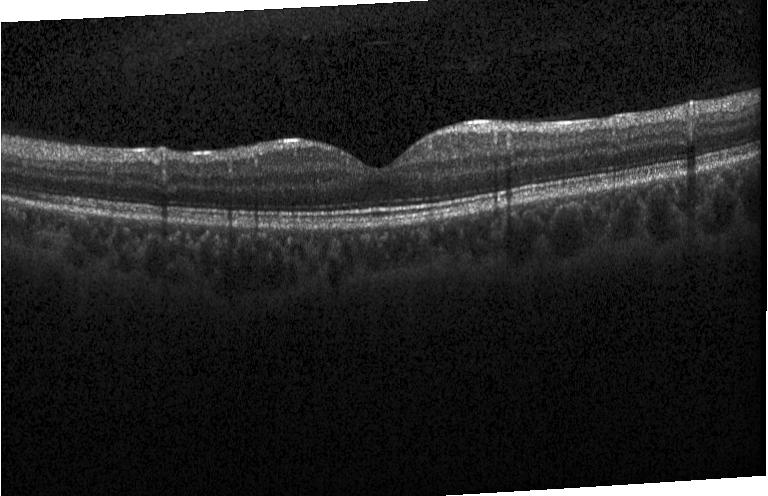

OCT line scan; Heidelberg Spectralis; horizontal scan through the fovea.
Finding: neither choroidal neovascularization, diabetic macular edema, nor drusen.